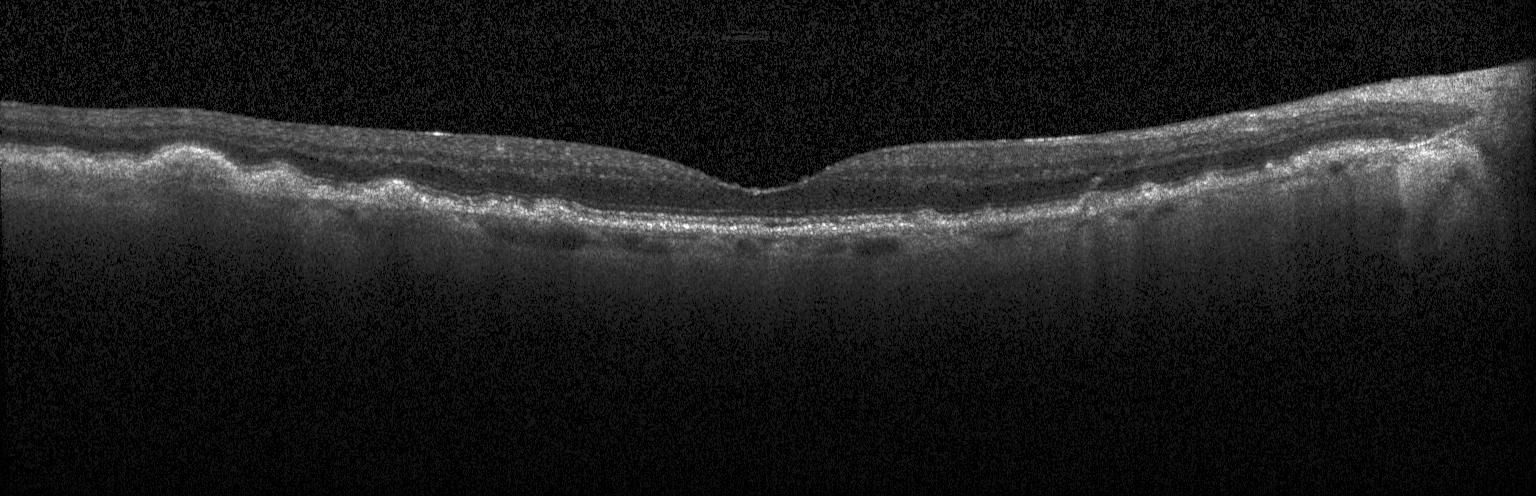

Retinal OCT cross-section. Acquired on a Heidelberg Spectralis
Sub-RPE drusenoid deposits.